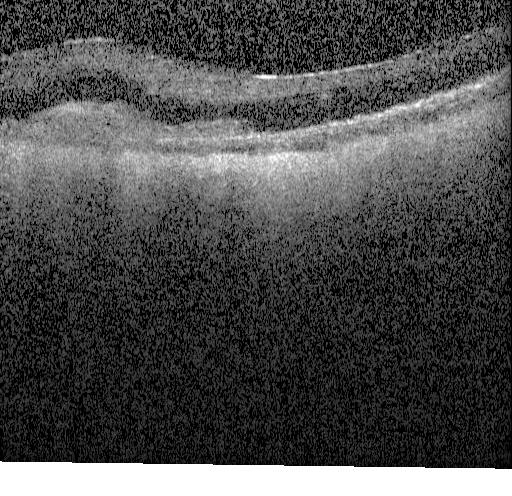 OCT finding: a choroidal neovascular membrane.